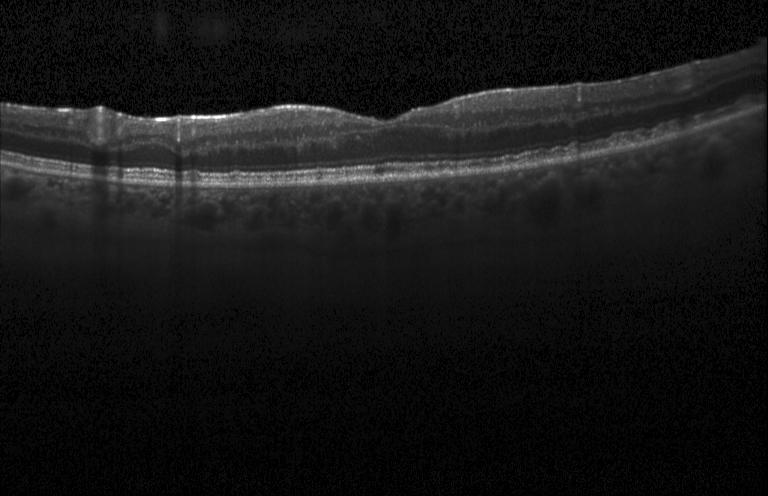 Optical coherence tomography scan. The scan shows drusen.